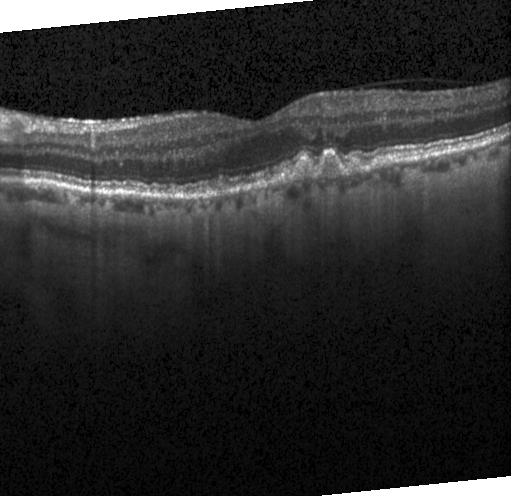
Retinal OCT B-scan
Impression: drusen.